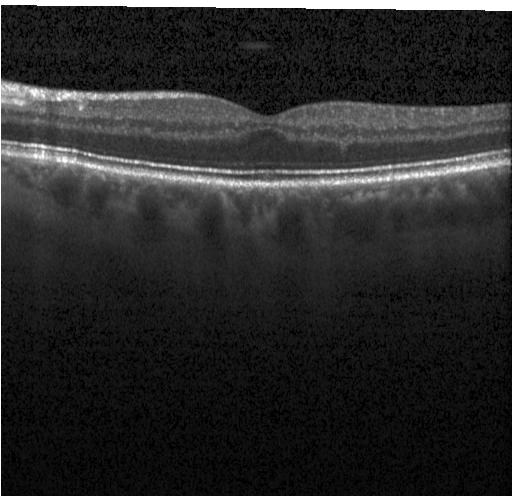
Impression: no choroidal neovascularization, no diabetic macular edema, and no drusen.